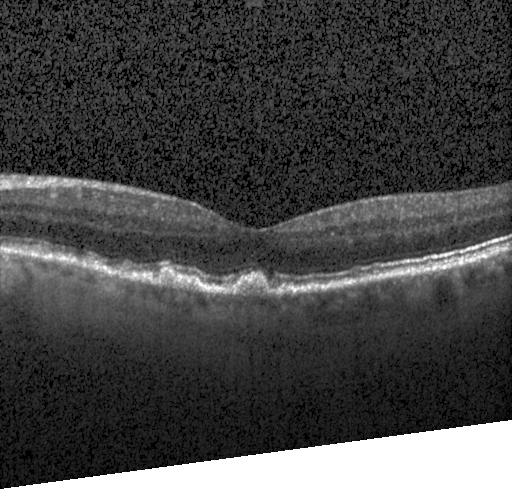
Retinal OCT cross-section
Diagnosis: drusen.